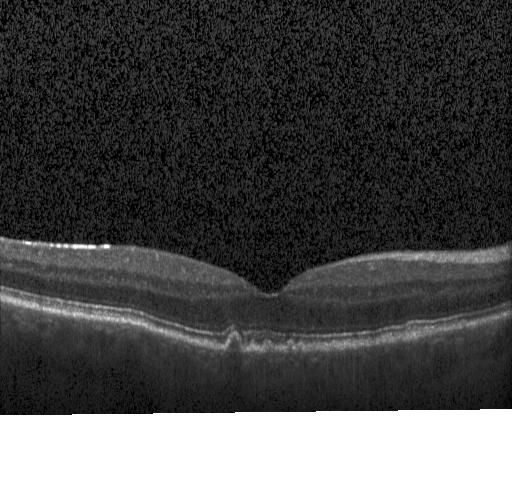

Macular scan · retinal OCT cross-section · spectral-domain OCT · Heidelberg Spectralis OCT system. Diagnosis: drusen.